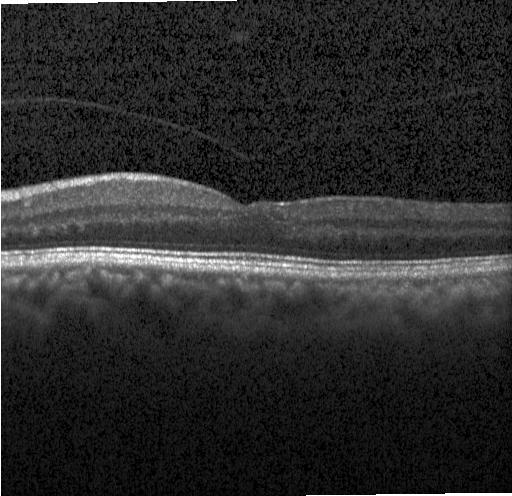
SD-OCT. OCT line scan.
Dx: no choroidal neovascularization, diabetic macular edema, or drusen.